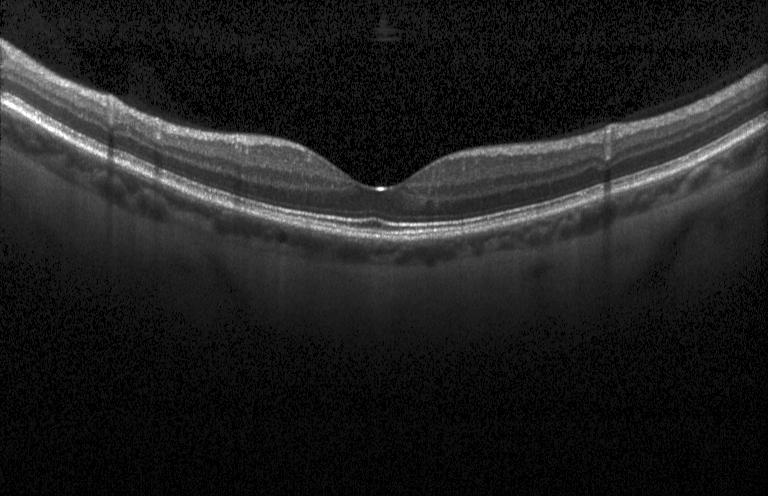

Spectral-domain optical coherence tomography; retinal OCT cross-section
Diagnosis: no CNV, no DME, and no drusen.